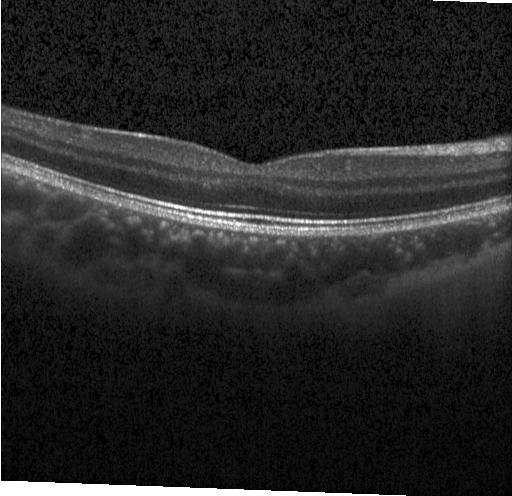

Diagnosis: no CNV, no DME, and no drusen.